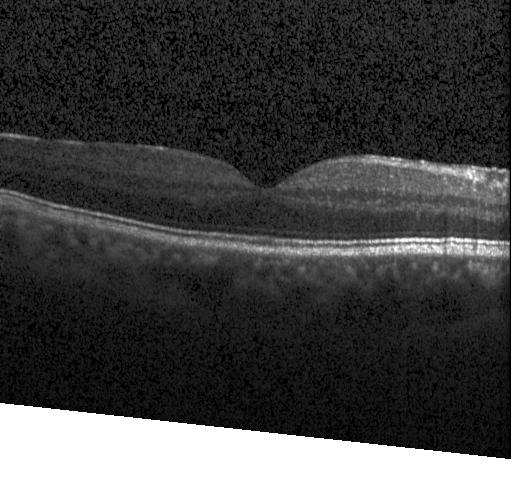 Spectral-domain optical coherence tomography; Heidelberg Spectralis OCT system; fovea-centered; optical coherence tomography B-scan.
Diagnosis: no choroidal neovascularization, no diabetic macular edema, and no drusen.